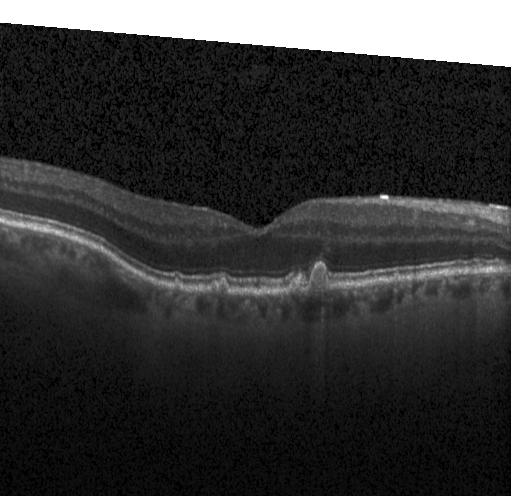 Spectral-domain optical coherence tomography; Heidelberg Spectralis OCT system; centered on the fovea; OCT B-scan — This B-scan demonstrates drusen.